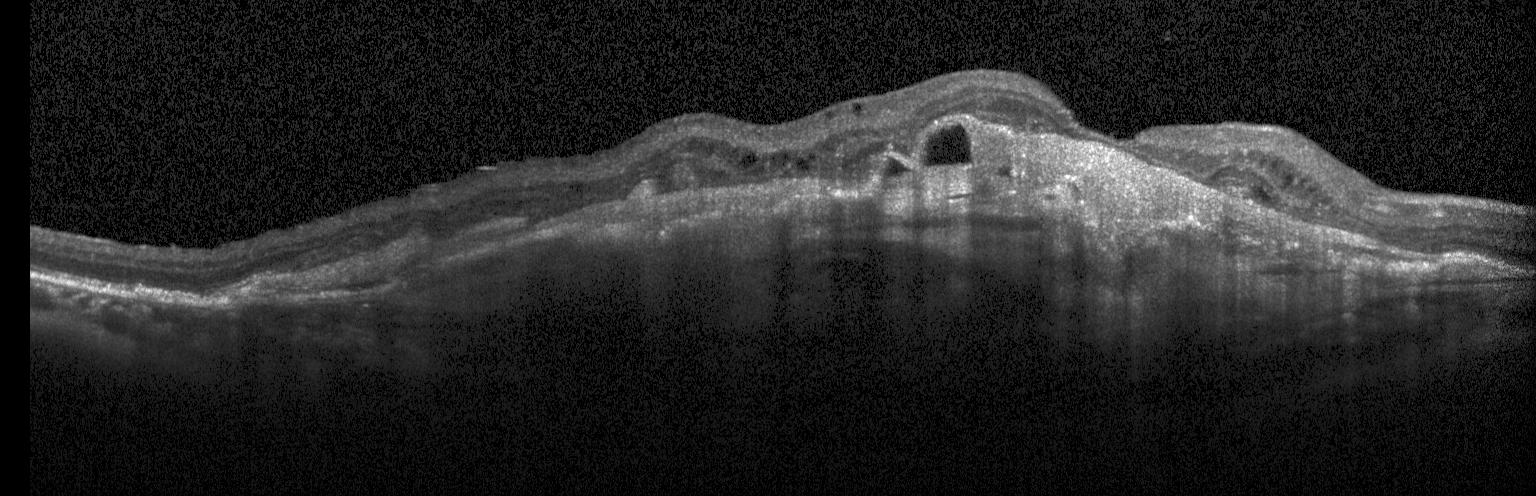 Optical coherence tomography B-scan; acquired on a Heidelberg Spectralis; centered on the fovea; spectral-domain OCT. The scan shows a choroidal neovascular membrane.